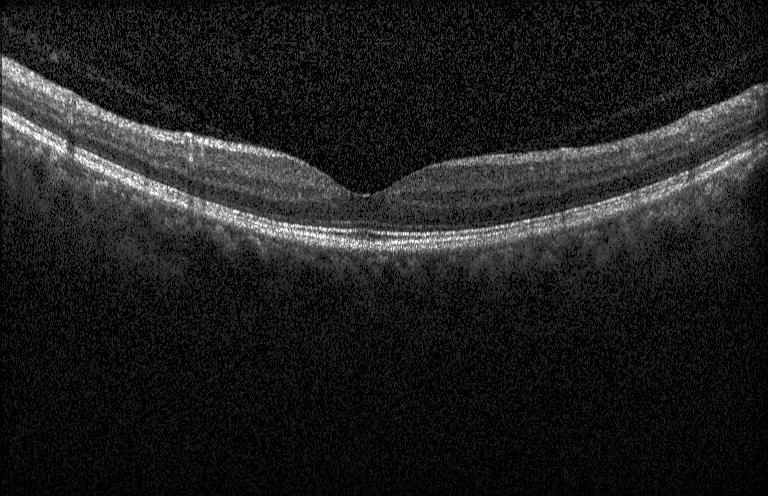
OCT scan showing neither CNV, DME, nor drusen.